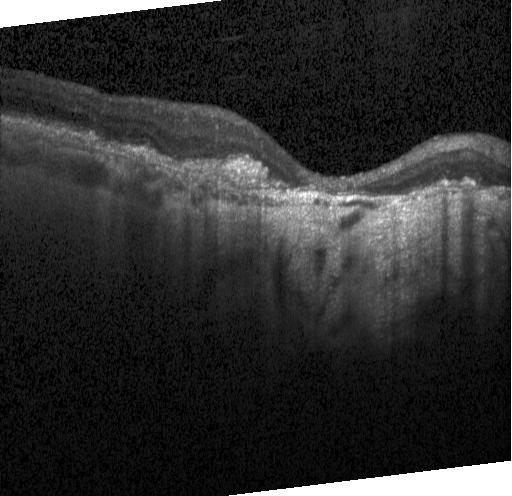

Instrument: Heidelberg Spectralis · spectral-domain optical coherence tomography · retinal OCT cross-section · macular scan
This B-scan demonstrates a choroidal neovascular membrane.